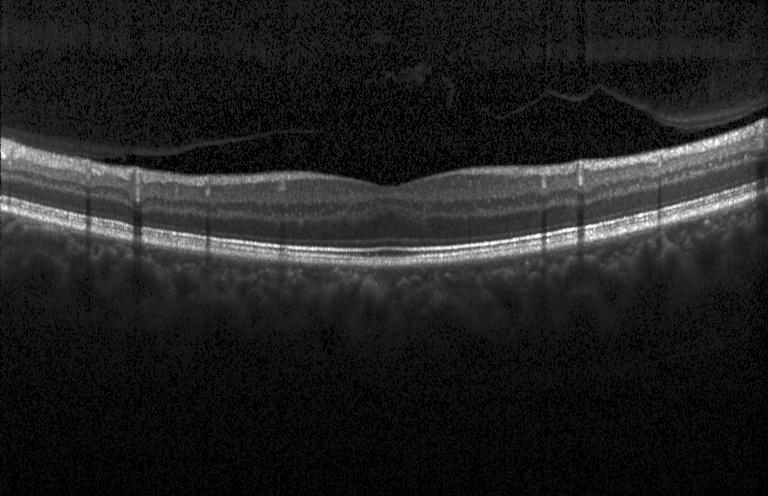
Finding: no evidence of CNV, DME, or drusen.